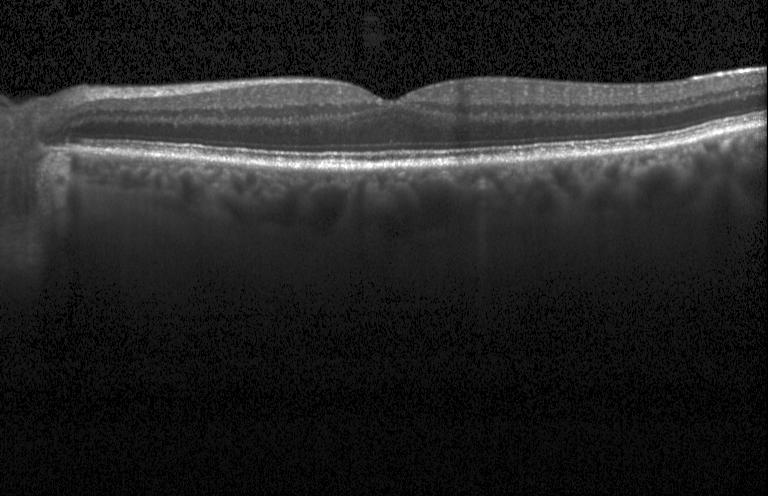
SD-OCT, horizontal scan through the fovea, optical coherence tomography B-scan — Impression: no choroidal neovascularization, no diabetic macular edema, and no drusen.